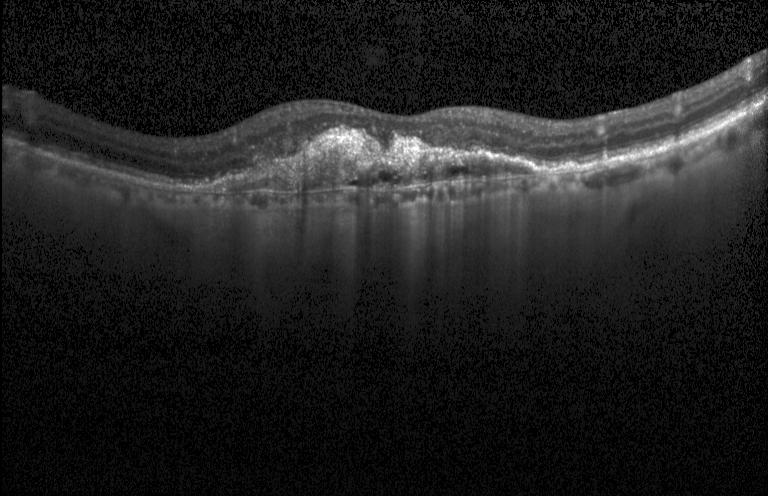
Spectral-domain optical coherence tomography. Retinal OCT B-scan. Through the macula
Finding: CNV.